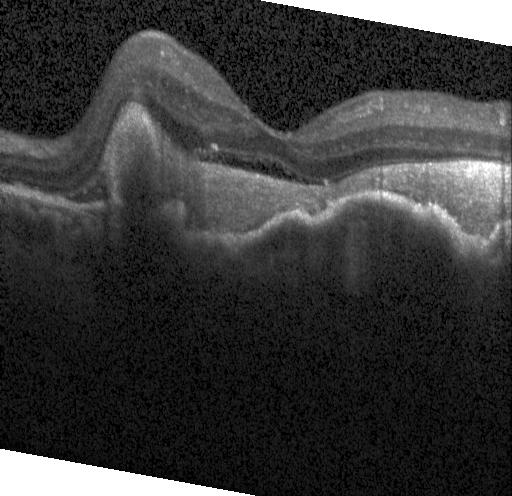

Finding: CNV.